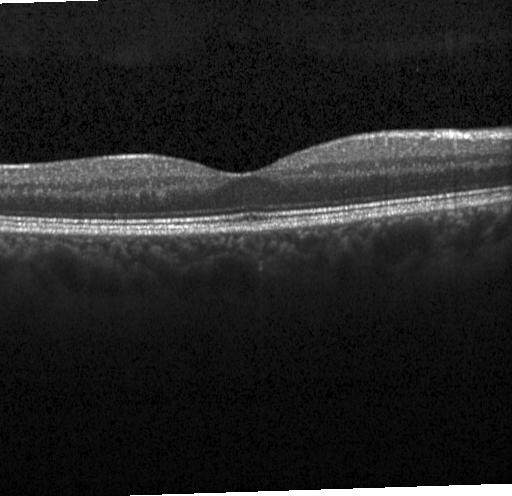

Dx: neither choroidal neovascularization, diabetic macular edema, nor drusen.